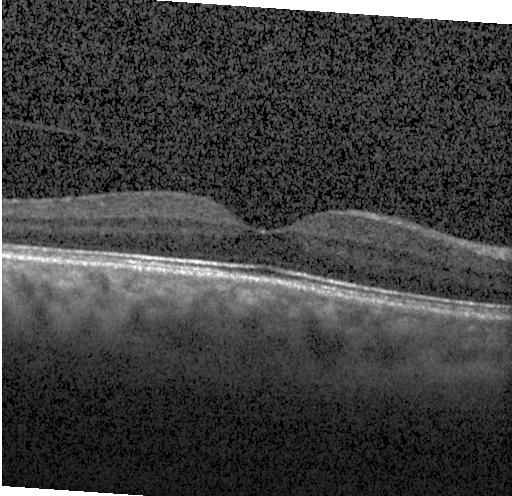
Spectral-domain optical coherence tomography; retinal OCT B-scan. This B-scan demonstrates no evidence of choroidal neovascularization, diabetic macular edema, or drusen.